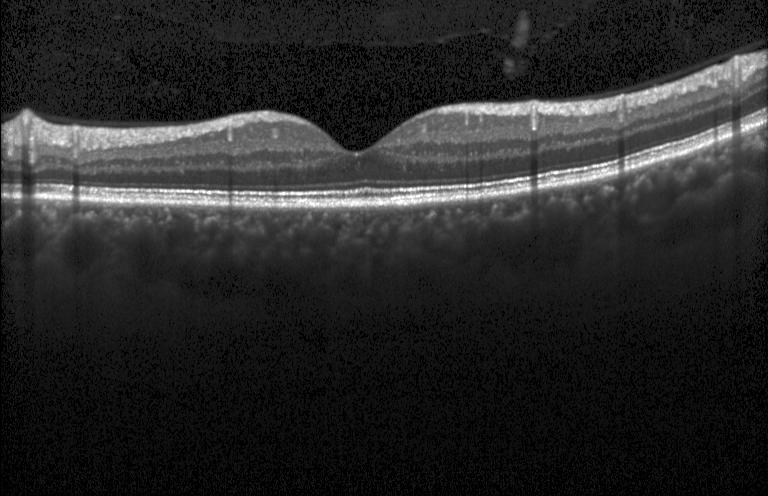
OCT B-scan showing no choroidal neovascularization, no diabetic macular edema, and no drusen.